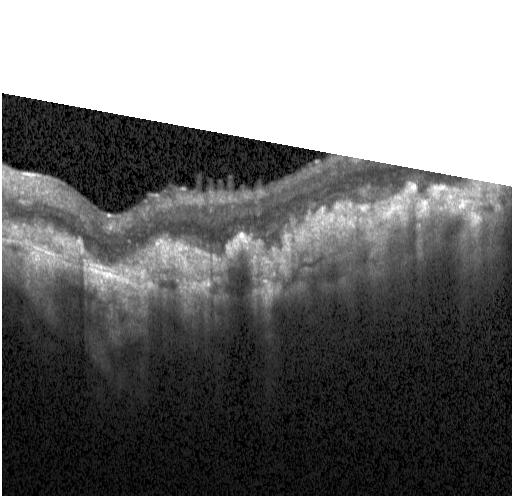 OCT line scan — OCT finding: choroidal neovascularization.